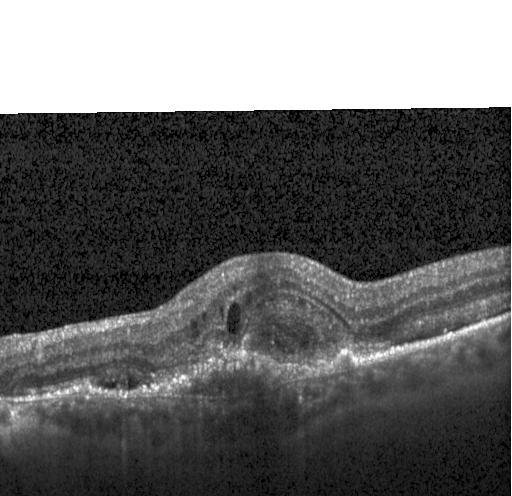 The scan shows a choroidal neovascular membrane.